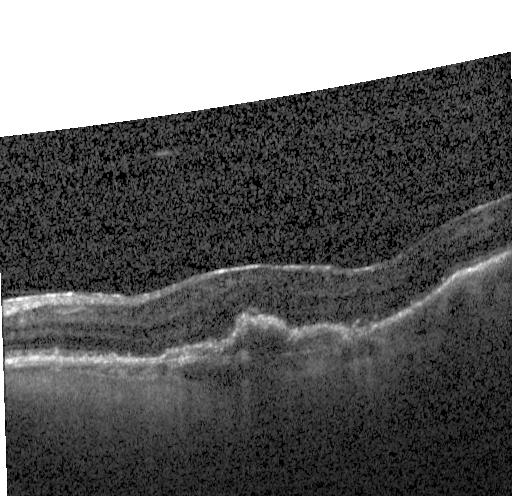 Fovea-centered; retinal OCT cross-section; instrument: Heidelberg Spectralis; spectral-domain OCT
This B-scan demonstrates a choroidal neovascular membrane.